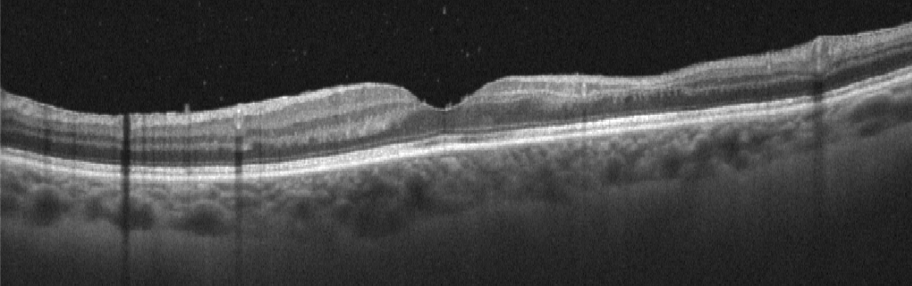

Retinal OCT B-scan — Dx: retinal vein occlusion.